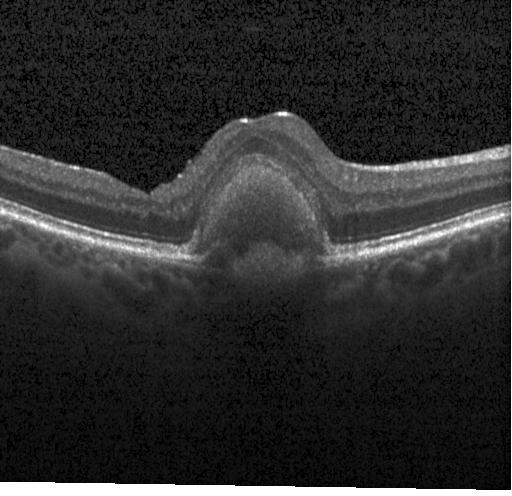
Finding: choroidal neovascularization.